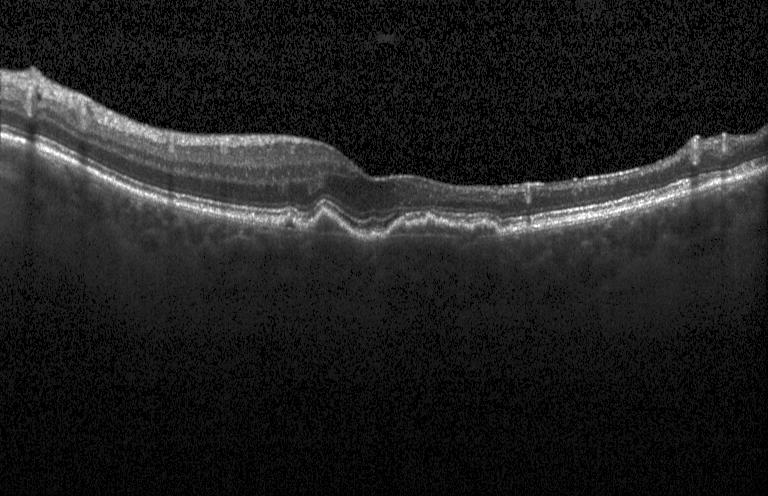

Spectral-domain optical coherence tomography. Instrument: Heidelberg Spectralis. Retinal OCT cross-section. Macular scan.
The scan shows a choroidal neovascular membrane.